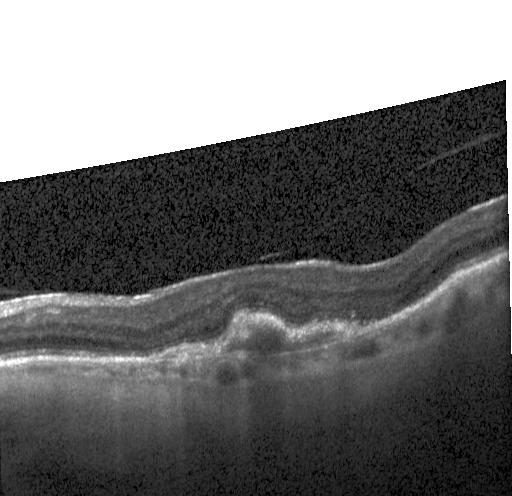 Dx: a choroidal neovascular membrane.